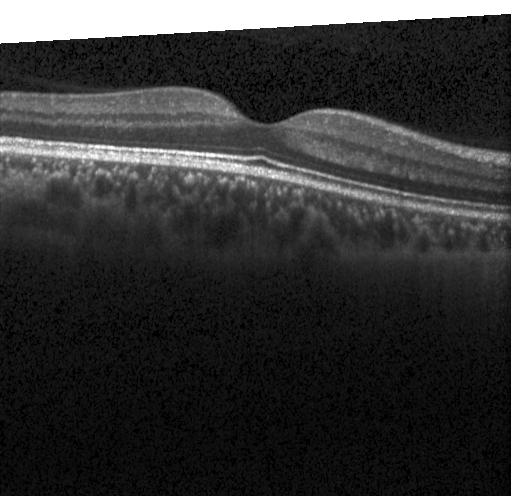
OCT scan showing neither choroidal neovascularization, diabetic macular edema, nor drusen.